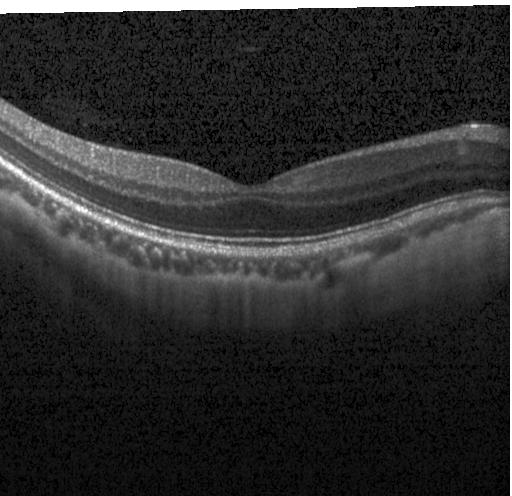
Optical coherence tomography scan. Finding: neither CNV, DME, nor drusen.